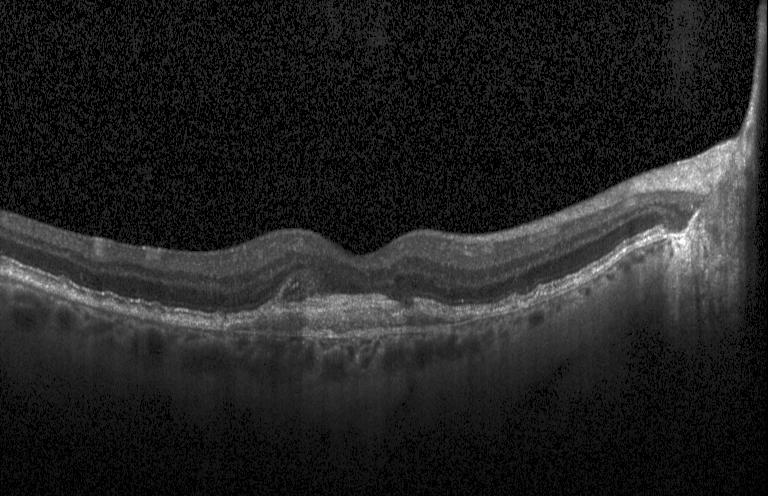 OCT scan showing choroidal neovascularization.